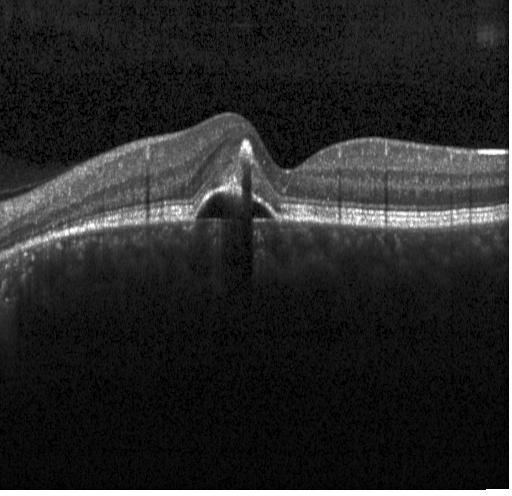
The scan shows a choroidal neovascular membrane.